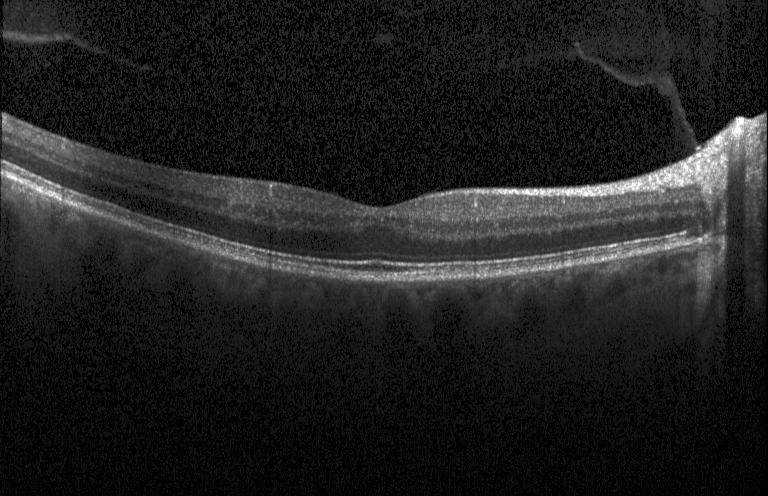
Retinal OCT B-scan; SD-OCT; horizontal scan through the fovea — The scan shows no choroidal neovascularization, diabetic macular edema, or drusen.